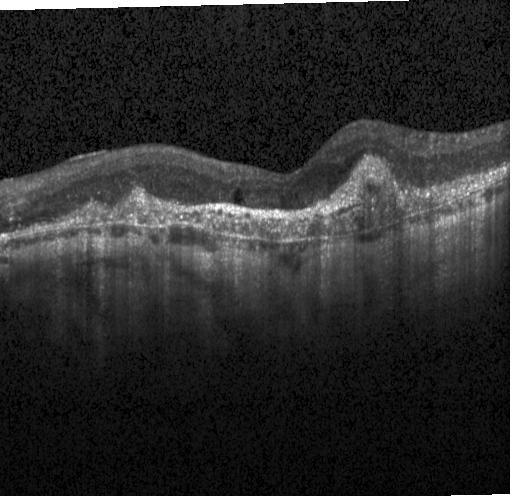

Diagnosis: CNV.